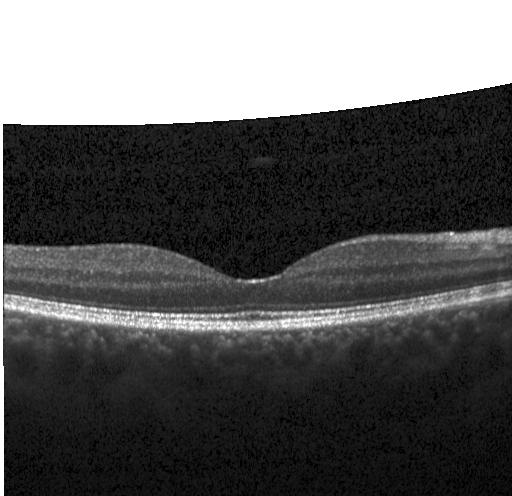 Through the macula, retinal OCT cross-section
Finding: no choroidal neovascularization, diabetic macular edema, or drusen.